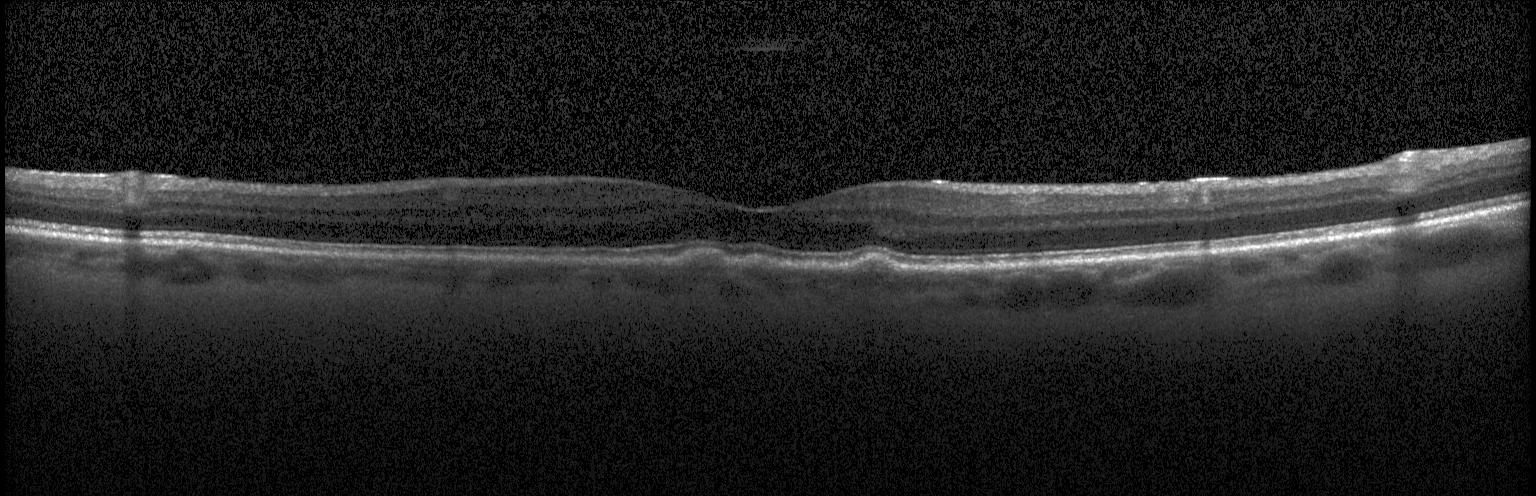

Finding: drusen.